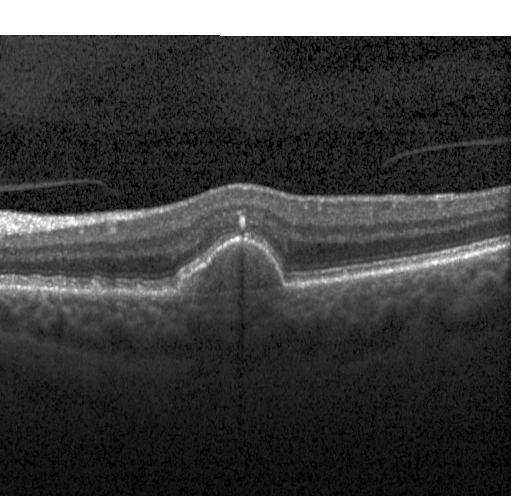
Centered on the fovea; retinal OCT cross-section; Heidelberg Spectralis OCT system; spectral-domain OCT
Diagnosis: choroidal neovascularization (CNV).